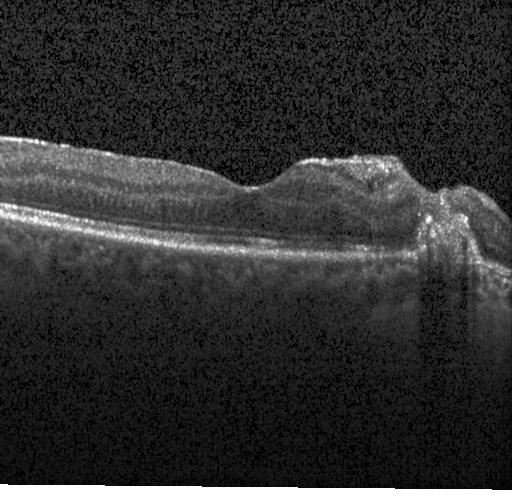 Fovea-centered · instrument: Heidelberg Spectralis · spectral-domain OCT · retinal OCT cross-section. This B-scan demonstrates choroidal neovascularization.